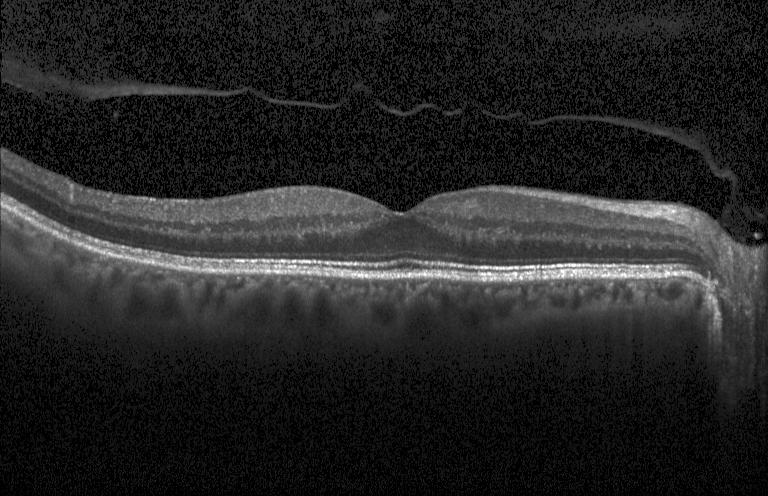
The scan shows no choroidal neovascularization, diabetic macular edema, or drusen.